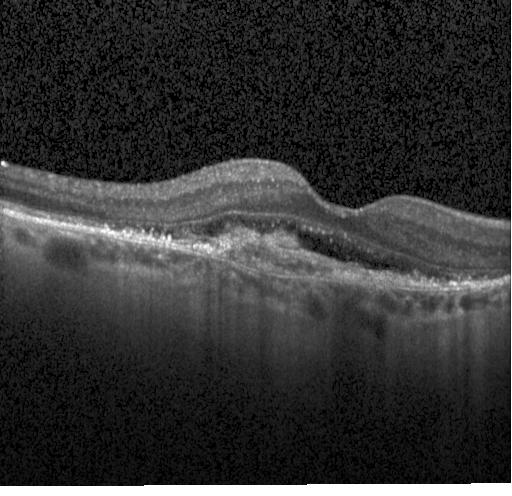
Heidelberg Spectralis, spectral-domain optical coherence tomography, OCT line scan, horizontal scan through the fovea
Impression: a choroidal neovascular membrane.